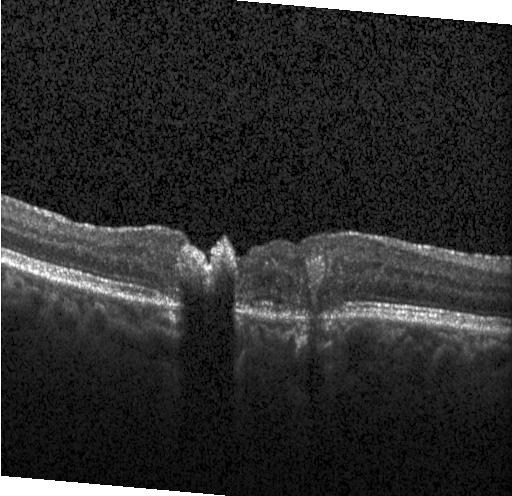 Through the macula. Optical coherence tomography B-scan. Heidelberg Spectralis — Choroidal neovascularization.